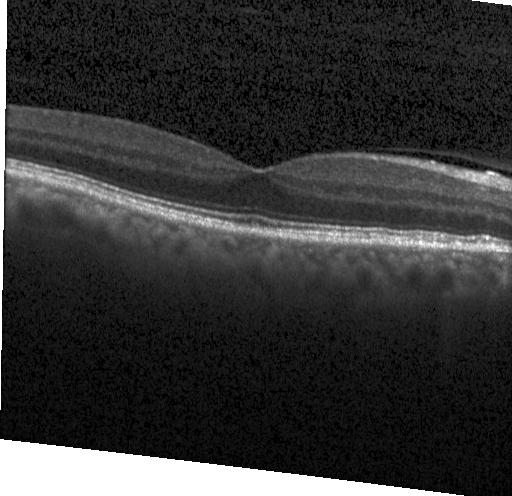 Spectral-domain optical coherence tomography; OCT line scan; centered on the fovea. Assessment: no evidence of choroidal neovascularization, diabetic macular edema, or drusen.